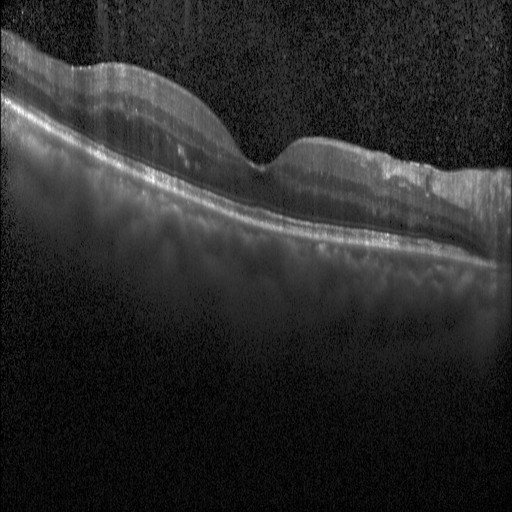

OCT line scan, through the macula, spectral-domain OCT. Impression: diabetic macular edema (DME).